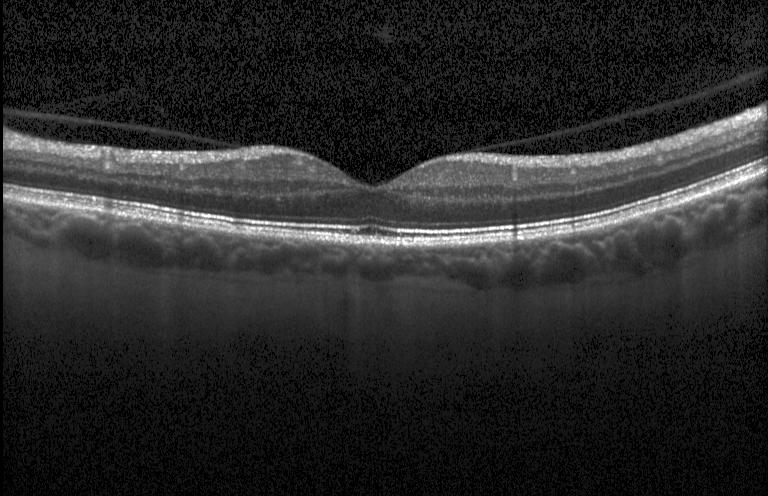 Retinal OCT cross-section showing no evidence of choroidal neovascularization, diabetic macular edema, or drusen.